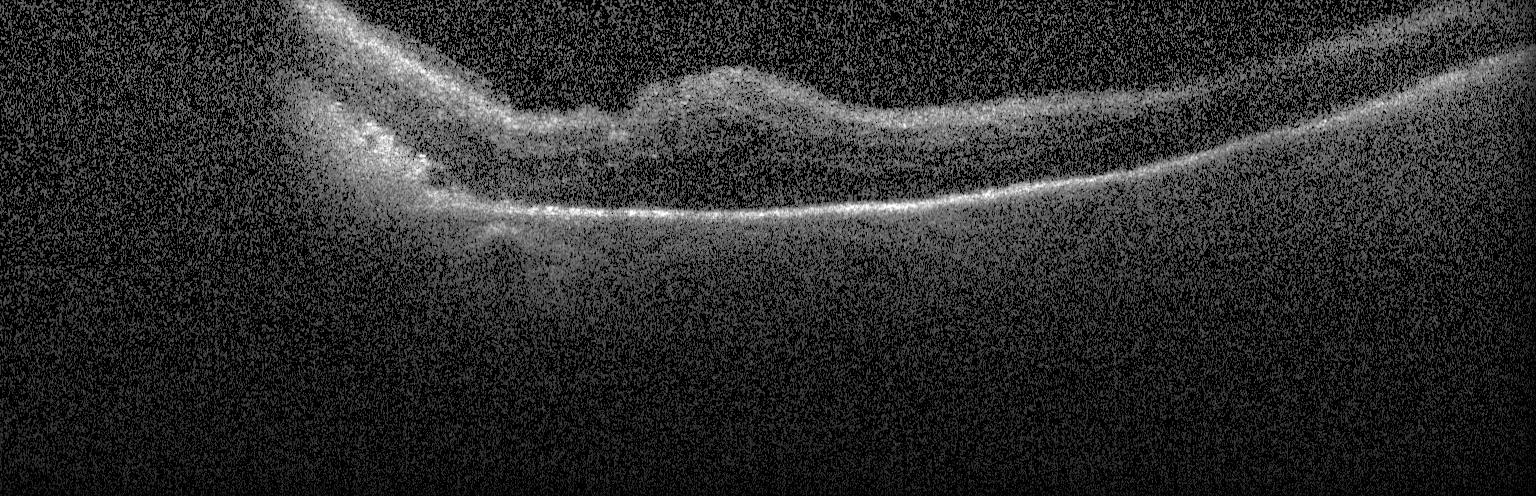
Optical coherence tomography scan; centered on the fovea; instrument: Heidelberg Spectralis; spectral-domain optical coherence tomography.
Impression: diabetic macular edema.